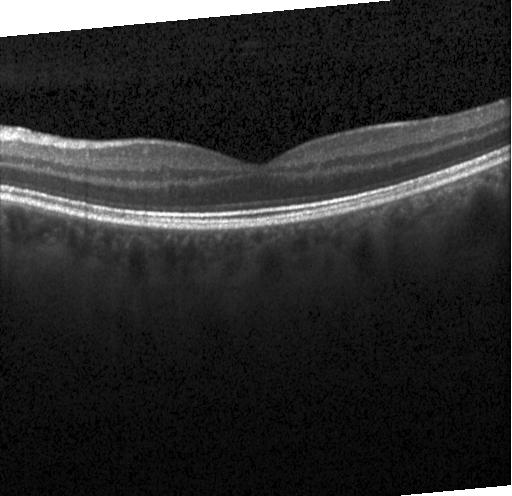

OCT scan showing no choroidal neovascularization, diabetic macular edema, or drusen.